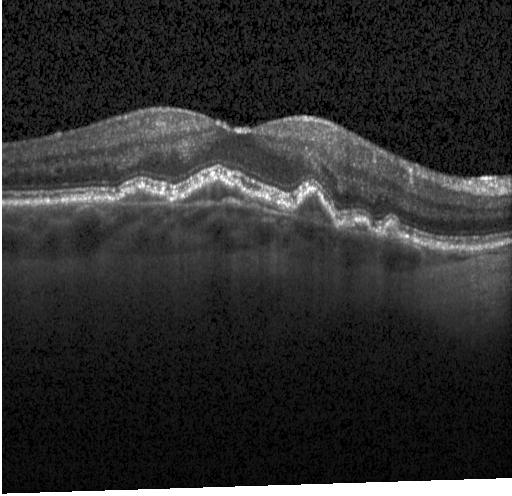
Dx: choroidal neovascularization (CNV).